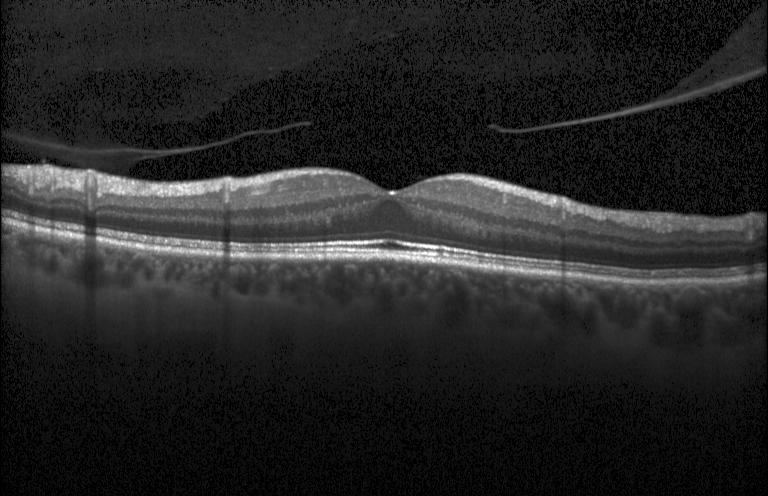 Assessment: no evidence of choroidal neovascularization, diabetic macular edema, or drusen.